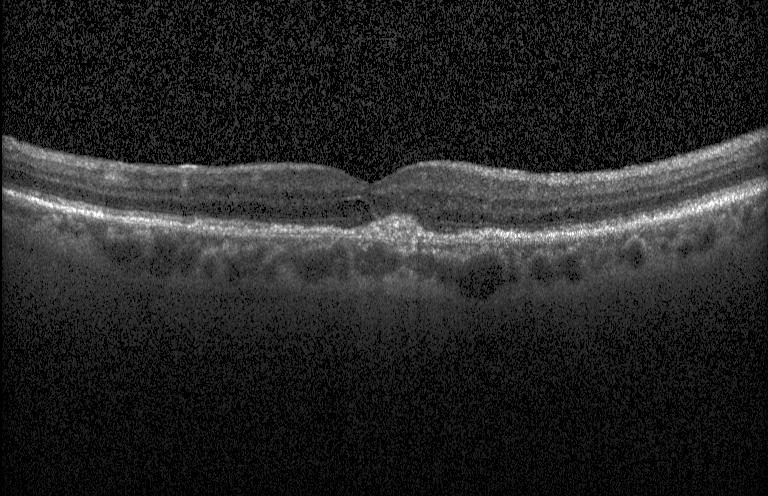
Assessment: choroidal neovascularization (CNV).